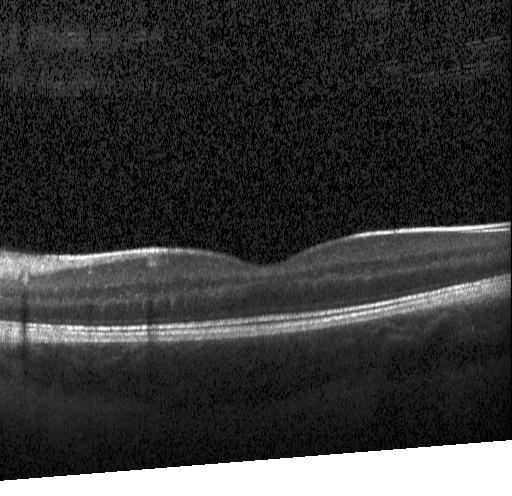 Spectral-domain OCT, retinal OCT cross-section.
Diagnosis: neither choroidal neovascularization, diabetic macular edema, nor drusen.